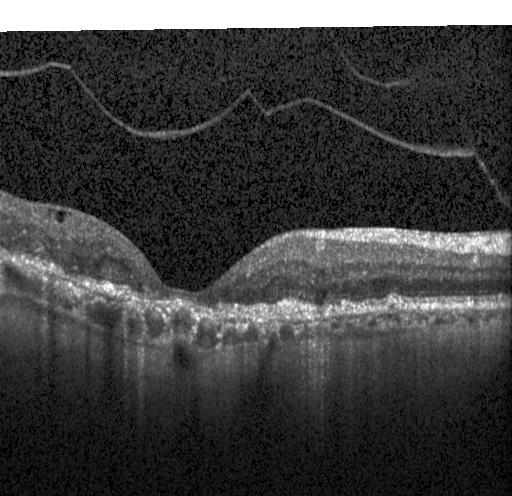
Finding: CNV.